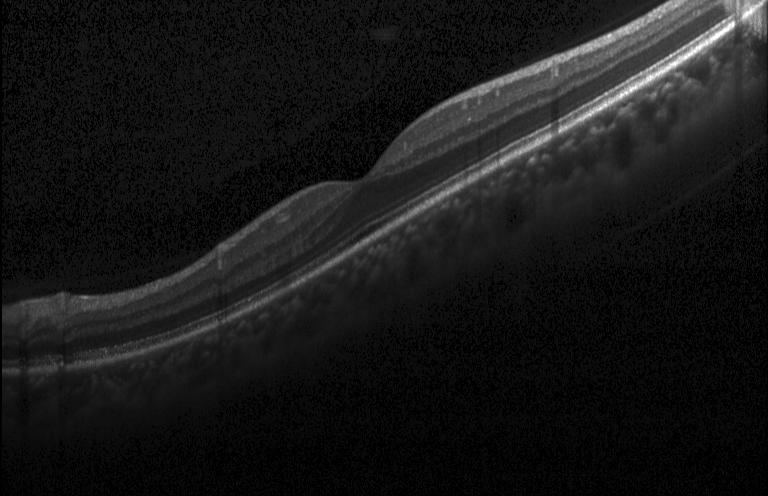 OCT line scan.
Macular OCT: no choroidal neovascularization, diabetic macular edema, or drusen.